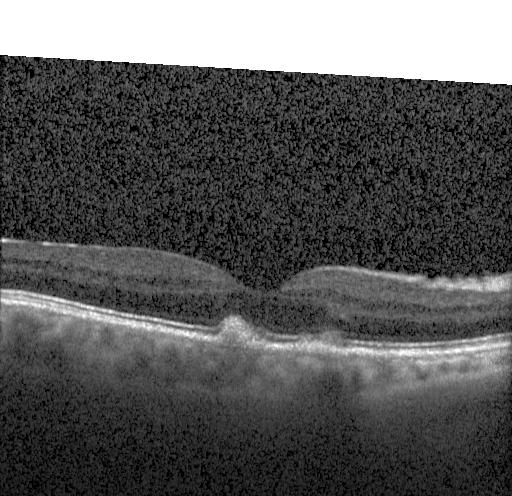 Optical coherence tomography B-scan
Finding: sub-RPE drusenoid deposits.